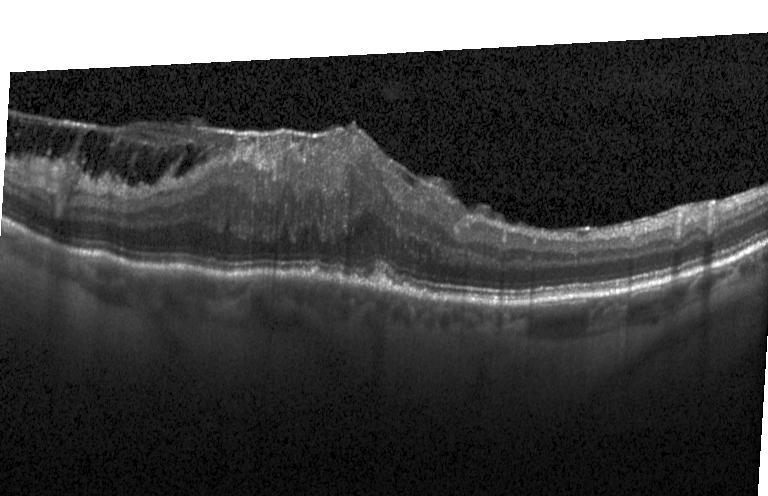

Retinal OCT B-scan — Diagnosis: drusen.